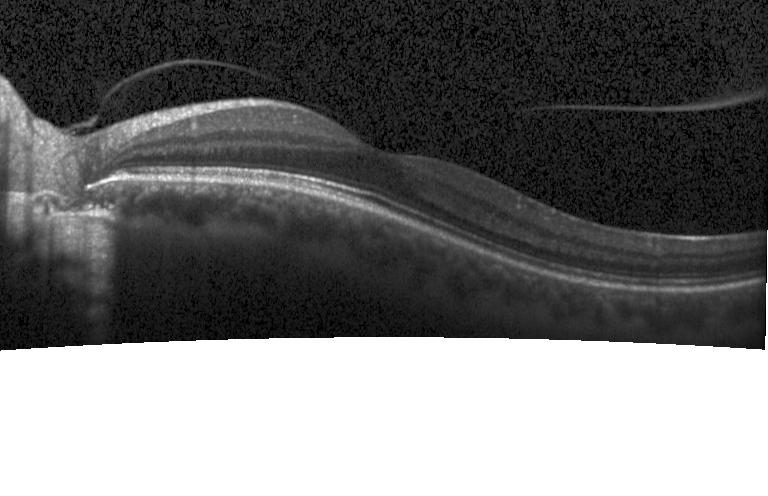 Through the macula. Retinal OCT B-scan — Assessment: neither CNV, DME, nor drusen.